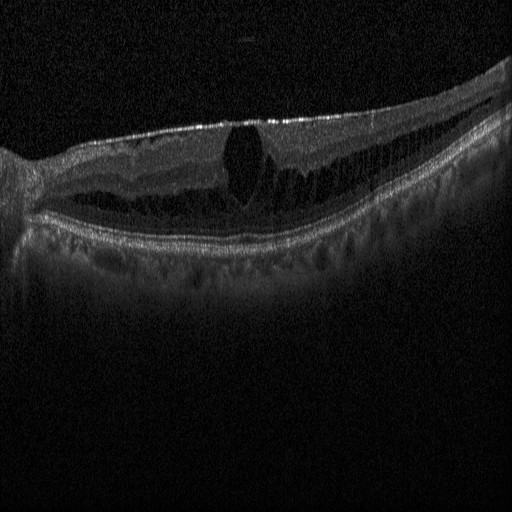

Optical coherence tomography scan
This B-scan demonstrates DME.